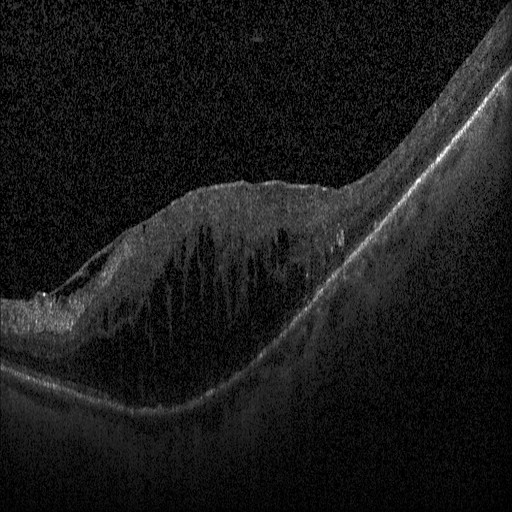

Macular scan · retinal OCT cross-section
Finding: diabetic macular edema.